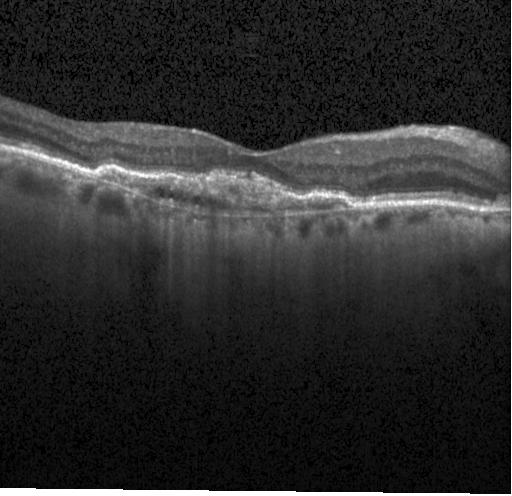 Spectral-domain OCT, instrument: Heidelberg Spectralis, retinal OCT B-scan, macular scan — Dx: a choroidal neovascular membrane.